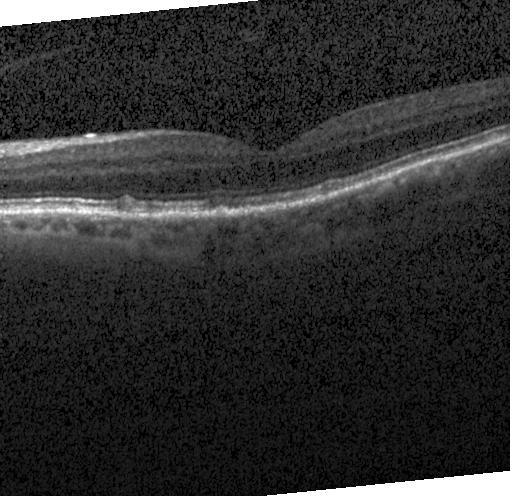 OCT B-scan showing drusen.